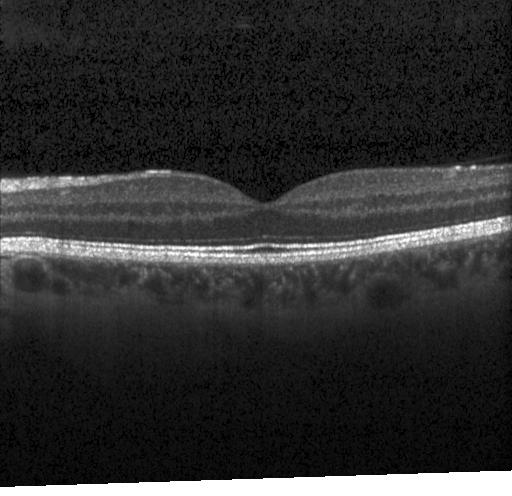
Retinal OCT B-scan; Heidelberg Spectralis OCT system; SD-OCT; fovea-centered
Finding: no CNV, no DME, and no drusen.